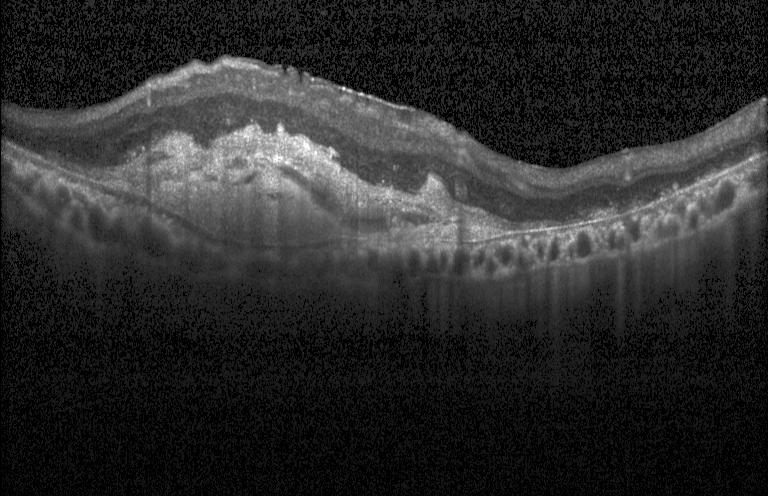 Macular OCT: choroidal neovascularization (CNV).